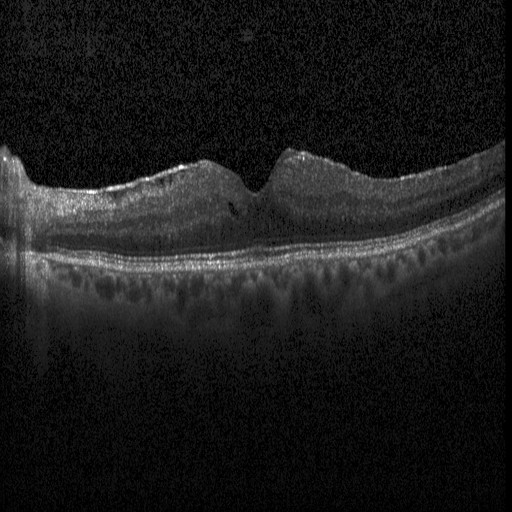

Spectral-domain optical coherence tomography. OCT line scan
Impression: diabetic macular edema (DME).